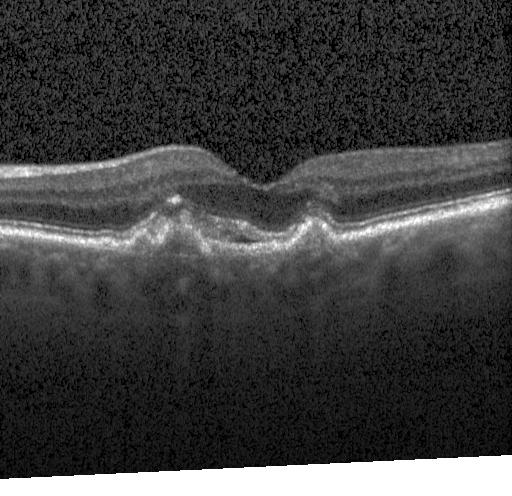

Diagnosis: choroidal neovascularization.